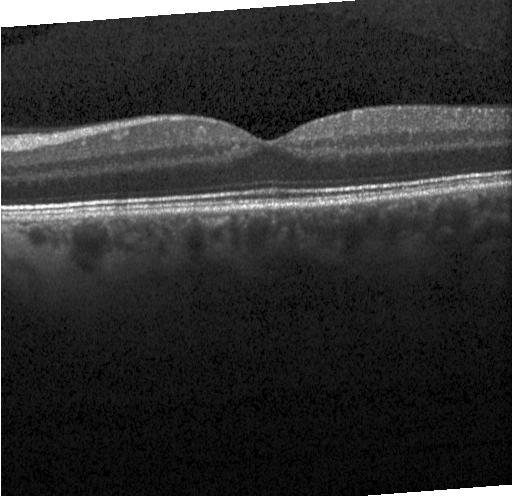 OCT B-scan; spectral-domain OCT.
No CNV, no DME, and no drusen.